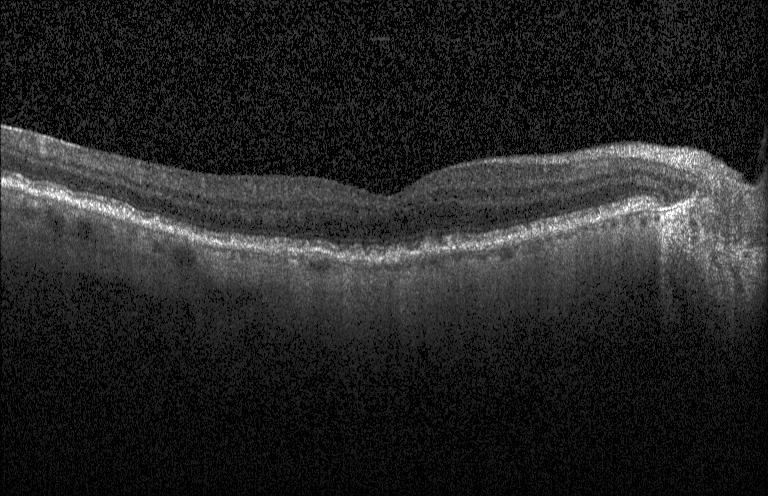

OCT B-scan · through the macula.
Impression: sub-RPE drusenoid deposits.